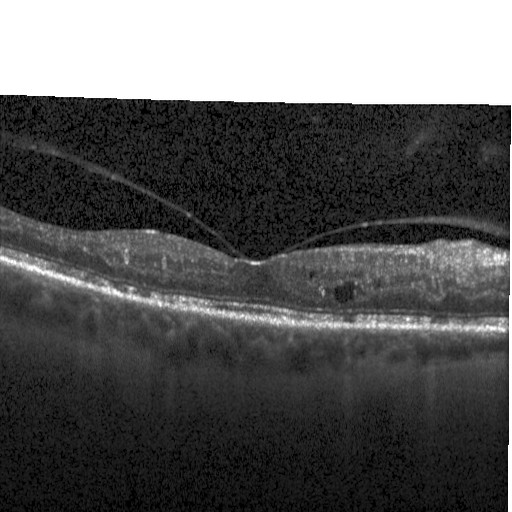
Retinal OCT cross-section.
Assessment: DME.